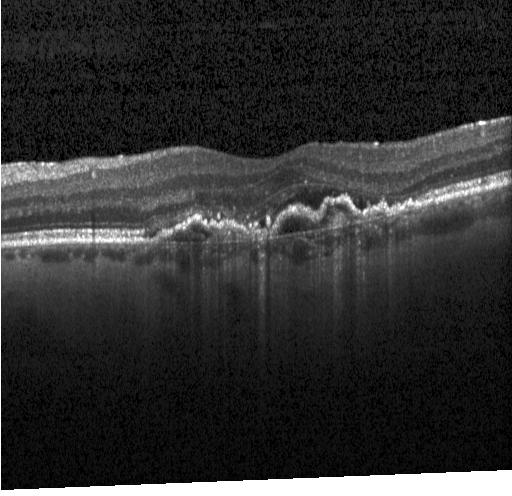 Impression: choroidal neovascularization (CNV).